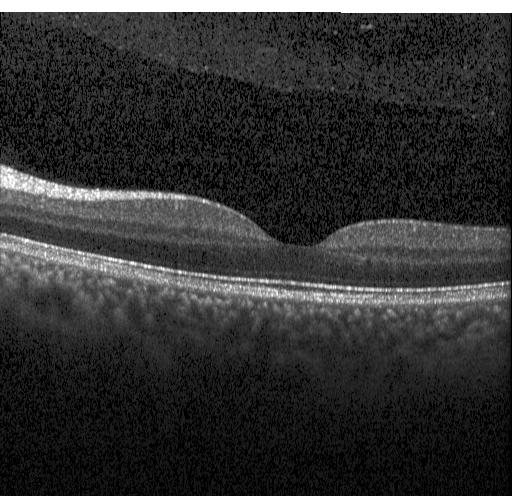

Horizontal scan through the fovea, Heidelberg Spectralis OCT system, optical coherence tomography B-scan.
This B-scan demonstrates neither choroidal neovascularization, diabetic macular edema, nor drusen.